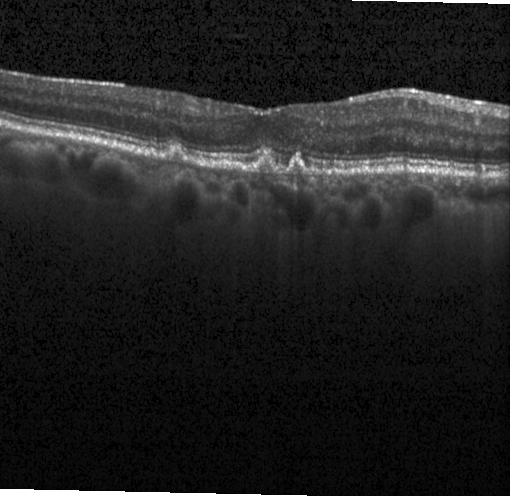 Finding: drusen.